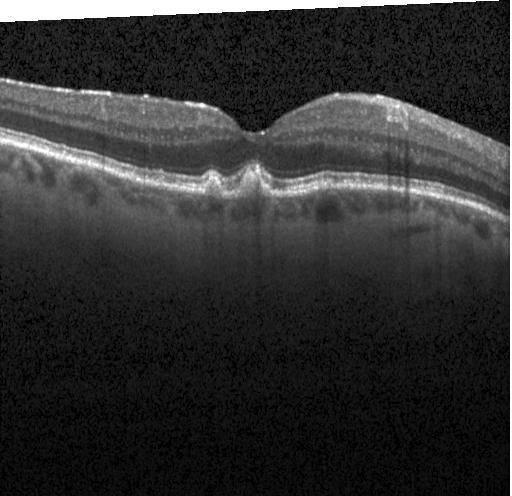
Optical coherence tomography B-scan · Heidelberg Spectralis OCT system. The scan shows drusen.